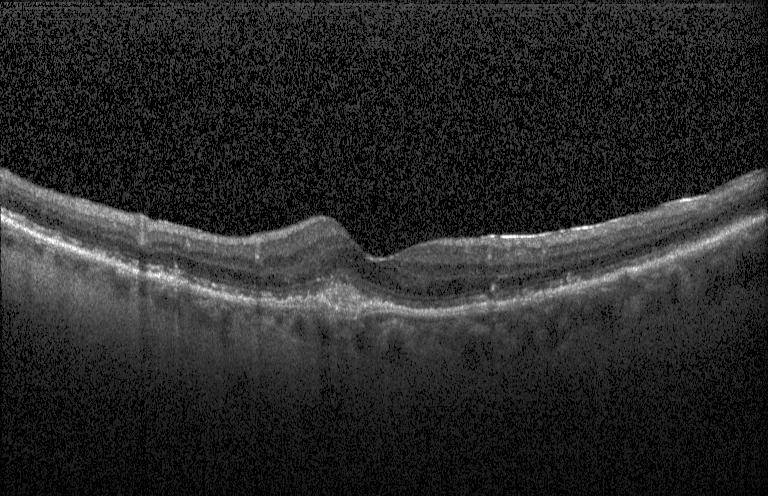
Diagnosis: a choroidal neovascular membrane.